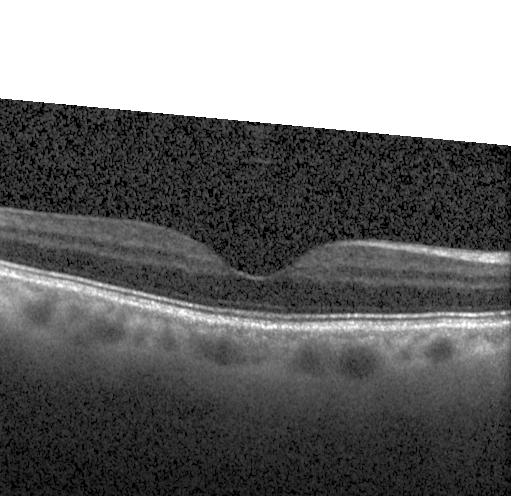 Spectral-domain OCT · through the macula · OCT B-scan · instrument: Heidelberg Spectralis.
Diagnosis: no evidence of choroidal neovascularization, diabetic macular edema, or drusen.